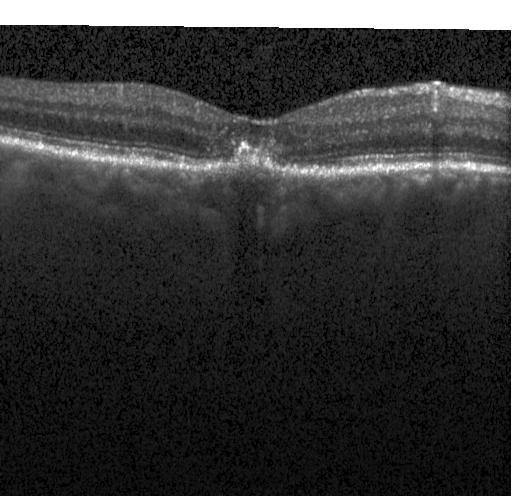 Spectral-domain optical coherence tomography. Heidelberg Spectralis. Retinal OCT cross-section. Through the macula.
Assessment: a choroidal neovascular membrane.